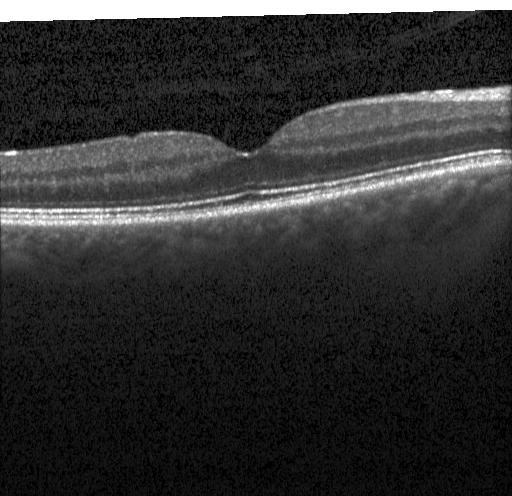 Retinal OCT cross-section, fovea-centered — Impression: no evidence of choroidal neovascularization, diabetic macular edema, or drusen.